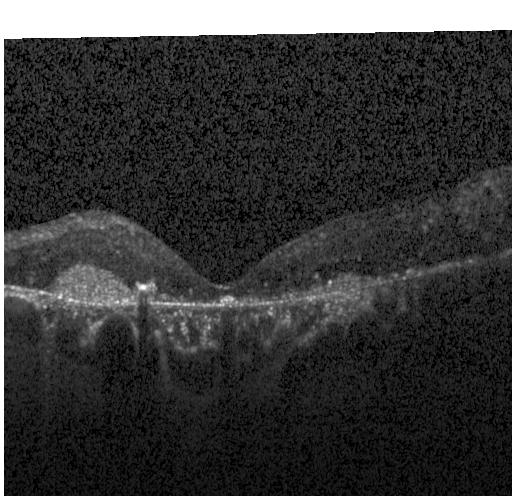 Diagnosis: a choroidal neovascular membrane.